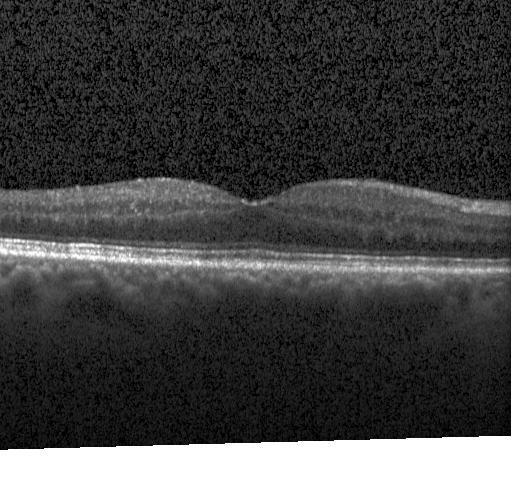
The scan shows no evidence of choroidal neovascularization, diabetic macular edema, or drusen.